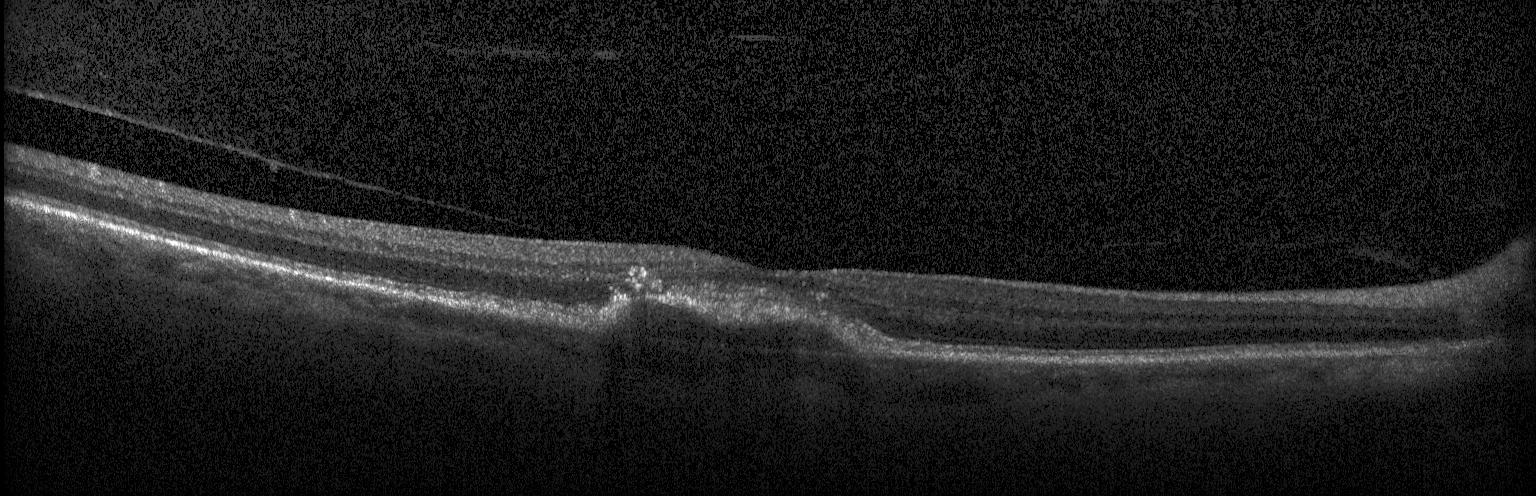
Spectral-domain optical coherence tomography. Centered on the fovea. Heidelberg Spectralis. Retinal OCT cross-section
Diagnosis: CNV.